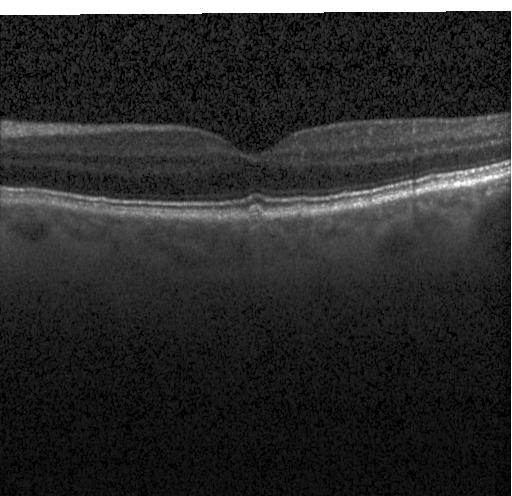

Retinal OCT cross-section. Assessment: drusen.